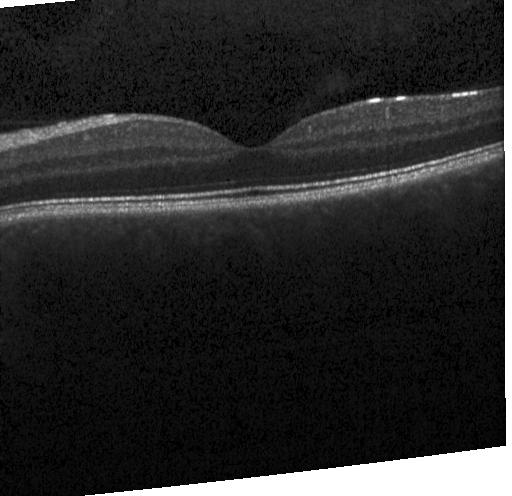

Acquired on a Heidelberg Spectralis, optical coherence tomography scan.
Diagnosis: neither CNV, DME, nor drusen.